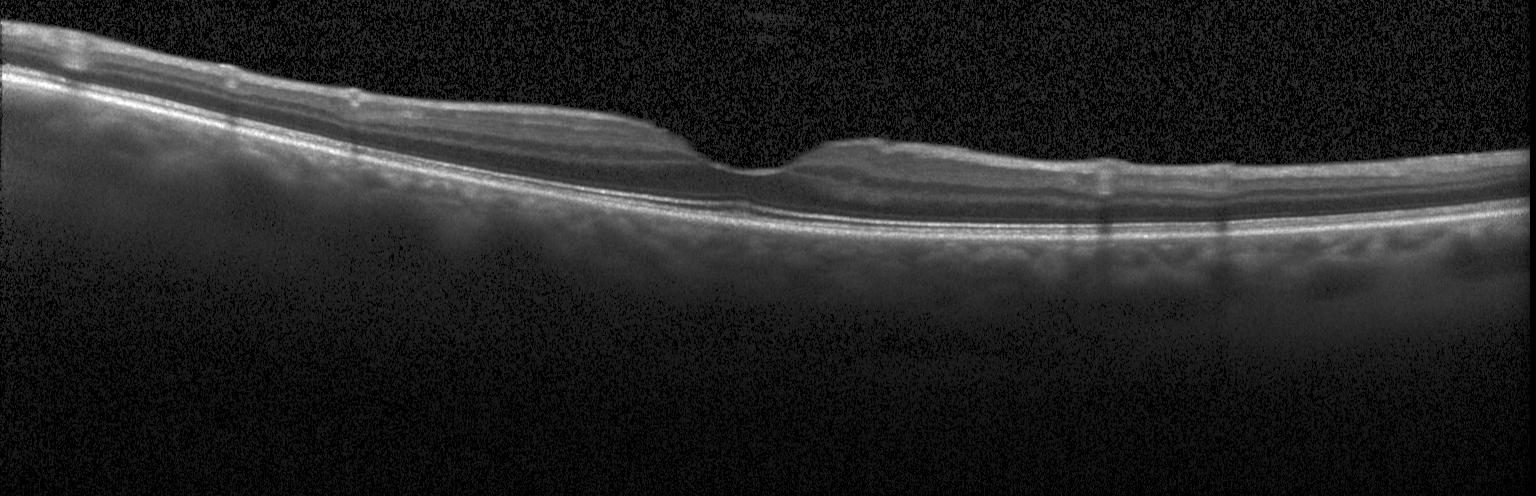

Retinal OCT B-scan · macular scan
Diagnosis: no evidence of CNV, DME, or drusen.